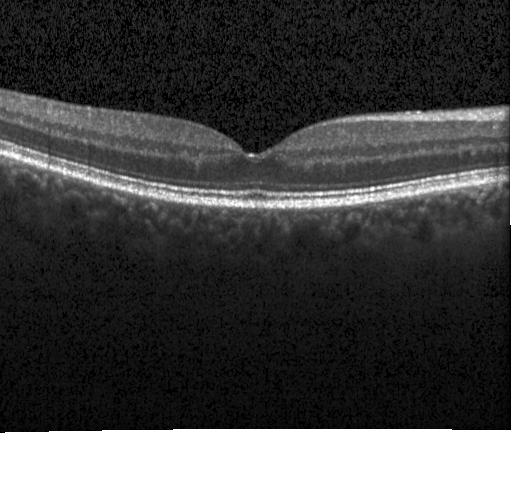
OCT B-scan showing no evidence of choroidal neovascularization, diabetic macular edema, or drusen.